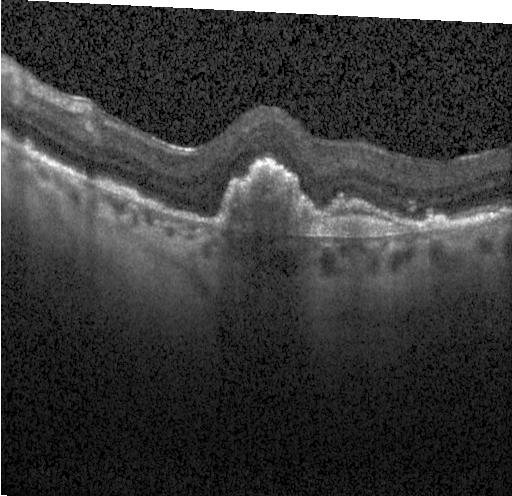

Macular OCT demonstrating a choroidal neovascular membrane.